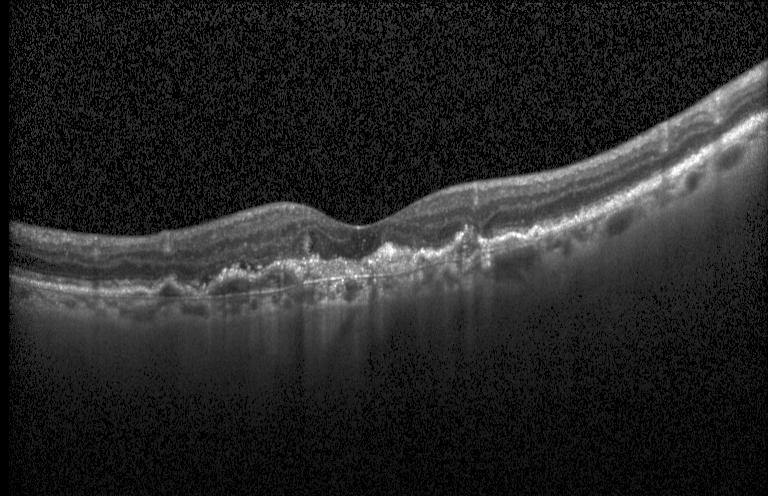

OCT B-scan, spectral-domain OCT, macular scan — Assessment: choroidal neovascularization (CNV).